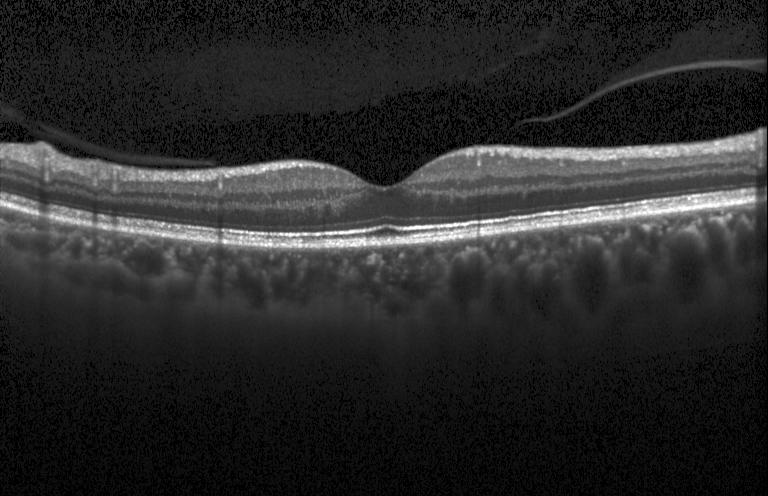
OCT B-scan
This B-scan demonstrates no CNV, DME, or drusen.